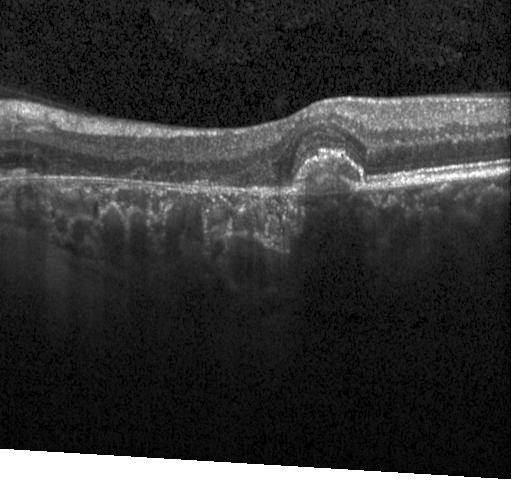
Acquired on a Heidelberg Spectralis, retinal OCT B-scan
Impression: a choroidal neovascular membrane.